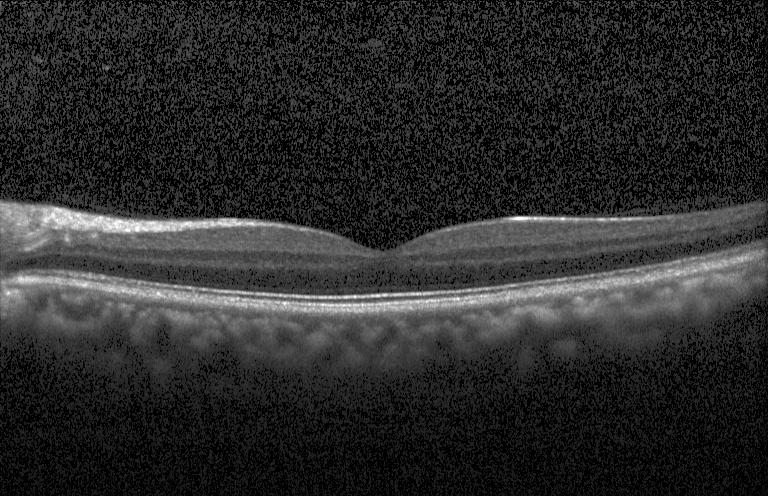
Assessment: no choroidal neovascularization, diabetic macular edema, or drusen.